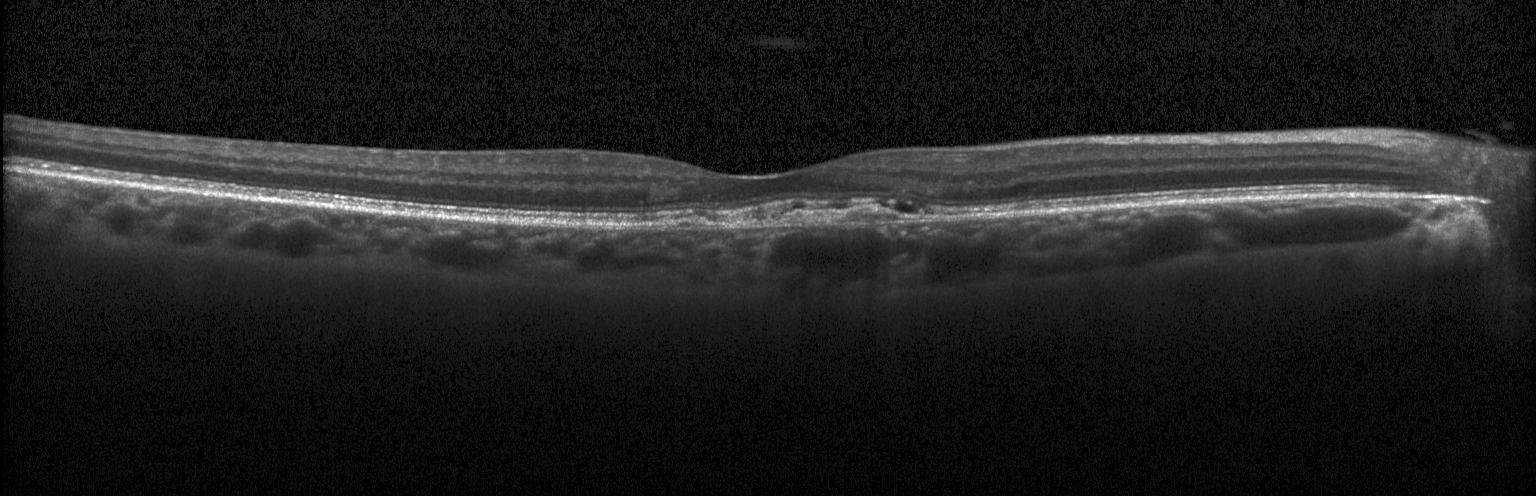 OCT scan showing choroidal neovascularization (CNV).